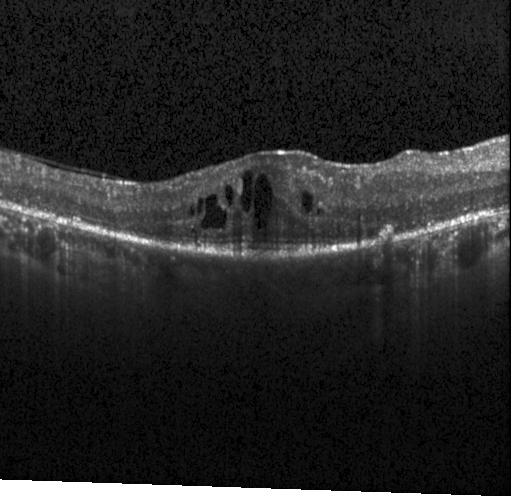
Retinal OCT cross-section. Heidelberg Spectralis OCT system. Horizontal scan through the fovea. Spectral-domain OCT. OCT finding: diabetic macular edema.